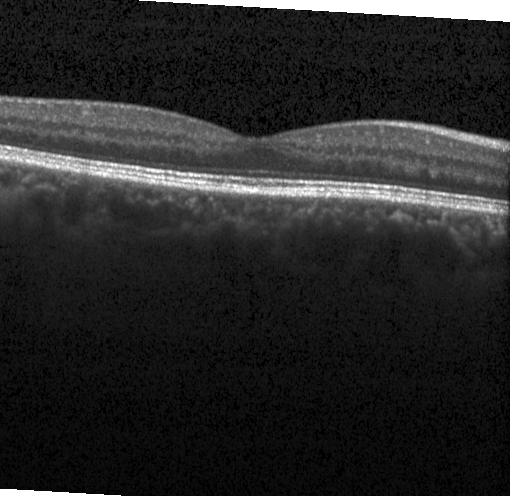 Instrument: Heidelberg Spectralis. Spectral-domain optical coherence tomography. Macular scan. OCT B-scan — OCT finding: no CNV, no DME, and no drusen.